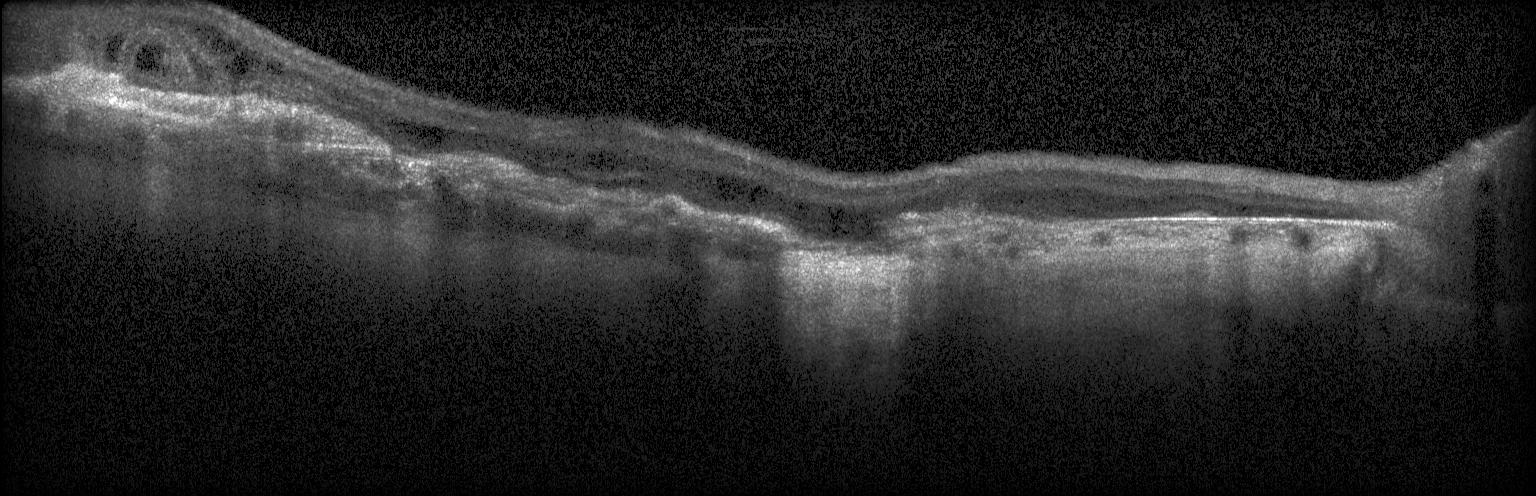 OCT B-scan; SD-OCT; centered on the fovea; Heidelberg Spectralis
Impression: a choroidal neovascular membrane.